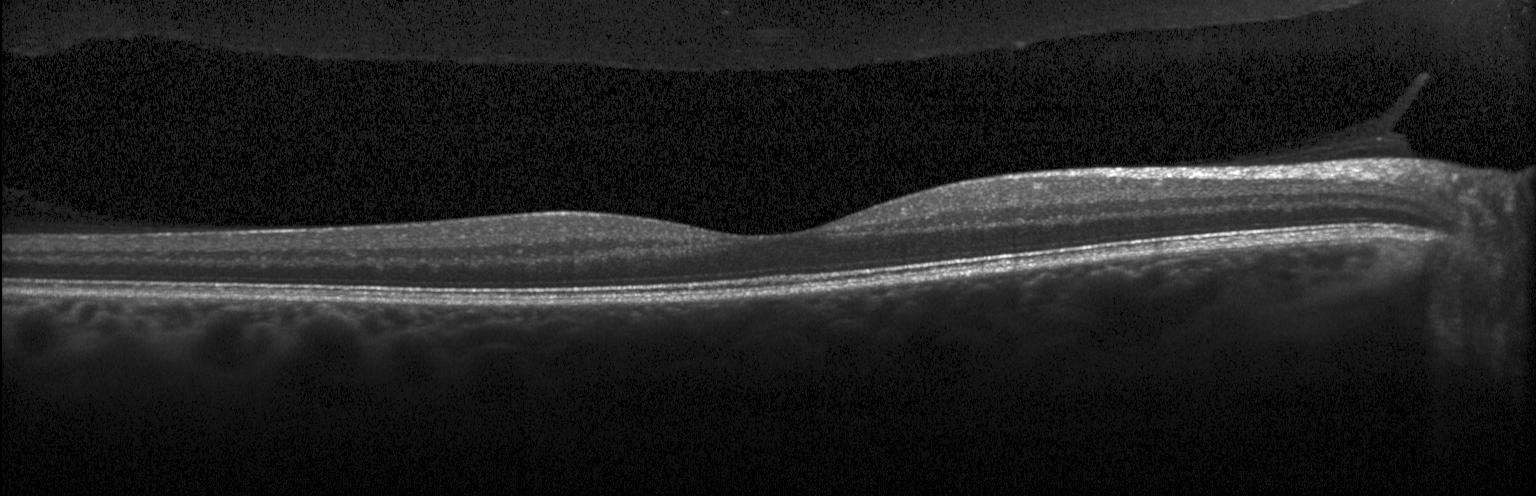
Retinal OCT B-scan
Finding: no choroidal neovascularization, no diabetic macular edema, and no drusen.